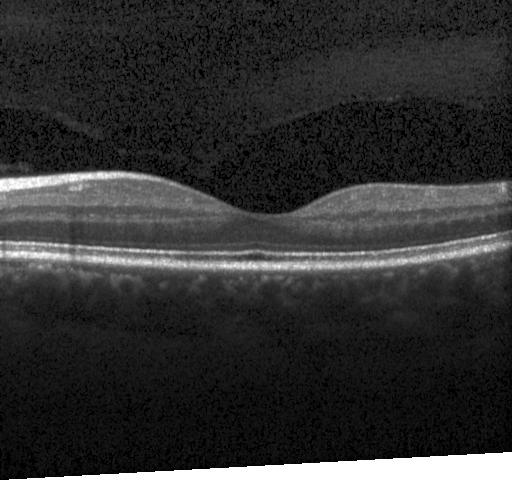
Optical coherence tomography scan; macular scan; Heidelberg Spectralis OCT system
No choroidal neovascularization, no diabetic macular edema, and no drusen.